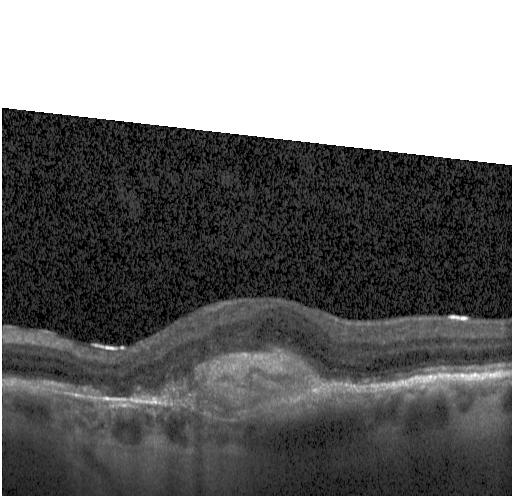

This B-scan demonstrates choroidal neovascularization (CNV).